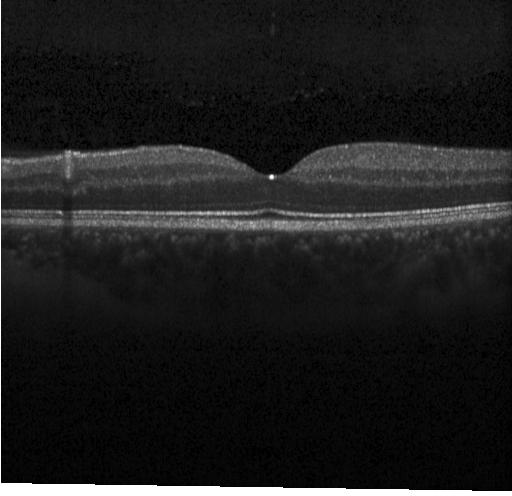

Spectral-domain optical coherence tomography. OCT B-scan. Through the macula.
Assessment: no choroidal neovascularization, diabetic macular edema, or drusen.